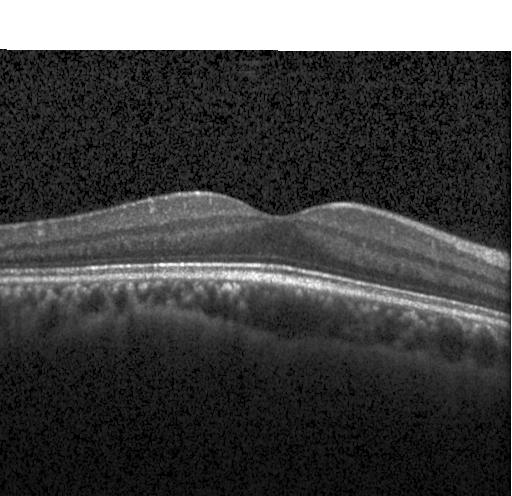
Macular scan; optical coherence tomography scan; spectral-domain optical coherence tomography.
Assessment: neither CNV, DME, nor drusen.